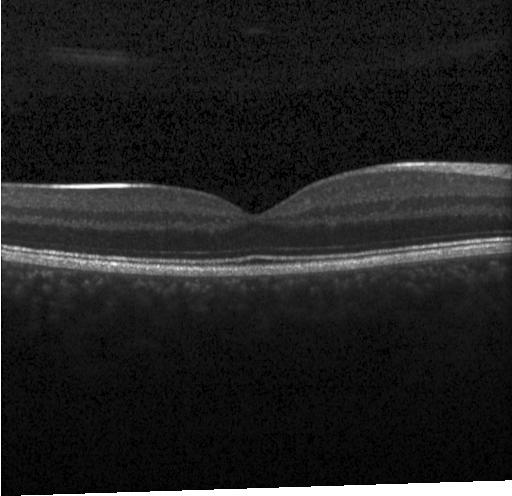

Impression: no CNV, DME, or drusen.